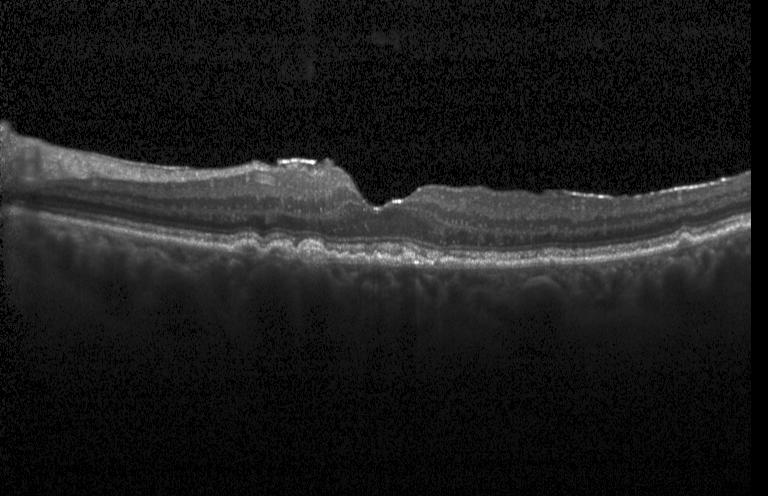 Retinal OCT B-scan; centered on the fovea. Finding: multiple drusen.